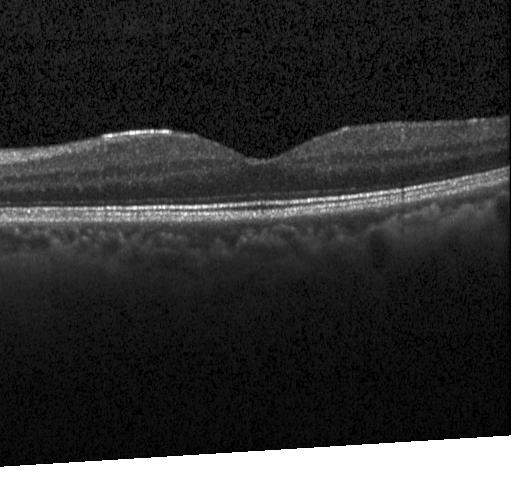 Diagnosis: no CNV, no DME, and no drusen.